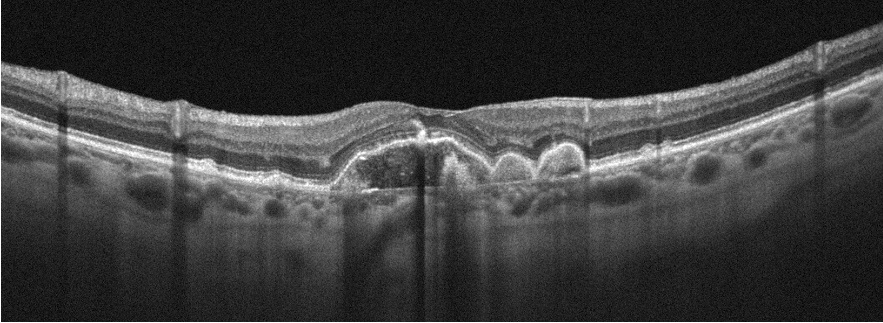 Through the macula · optical coherence tomography scan
Dx: age-related macular degeneration (AMD).